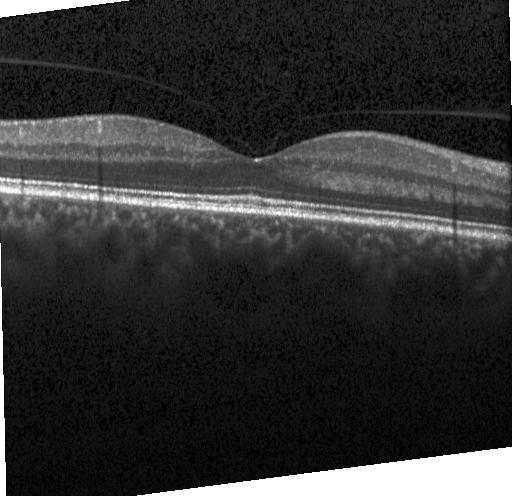 Macular OCT: no CNV, DME, or drusen.